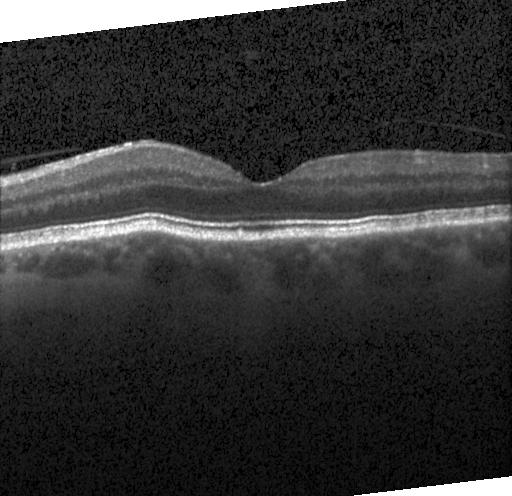
Macular OCT demonstrating no choroidal neovascularization, no diabetic macular edema, and no drusen.